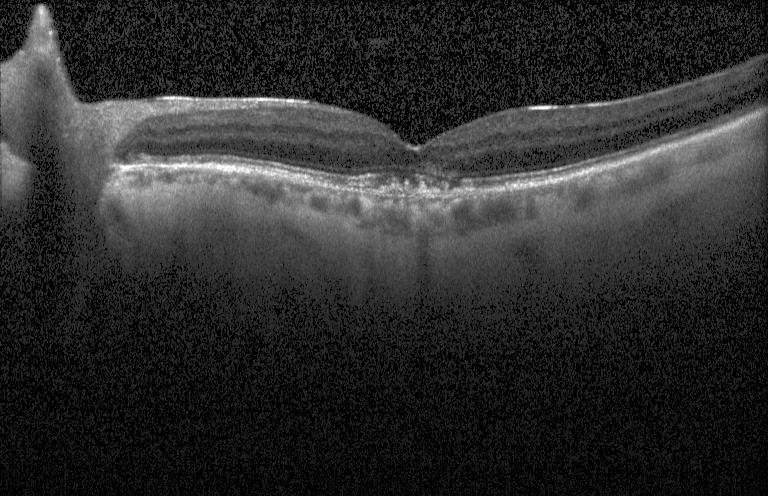
Assessment: CNV.